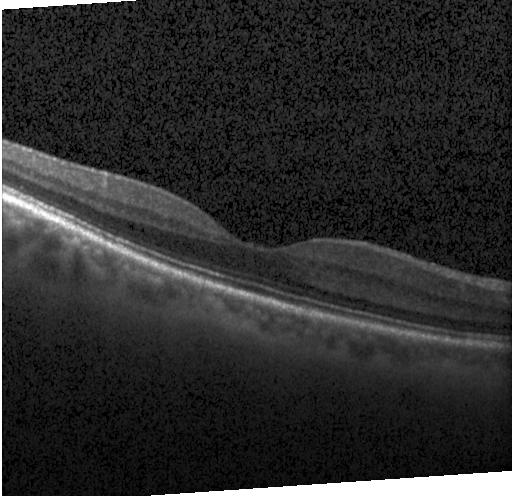
Horizontal scan through the fovea · spectral-domain optical coherence tomography · OCT line scan · acquired on a Heidelberg Spectralis — OCT finding: no CNV, no DME, and no drusen.